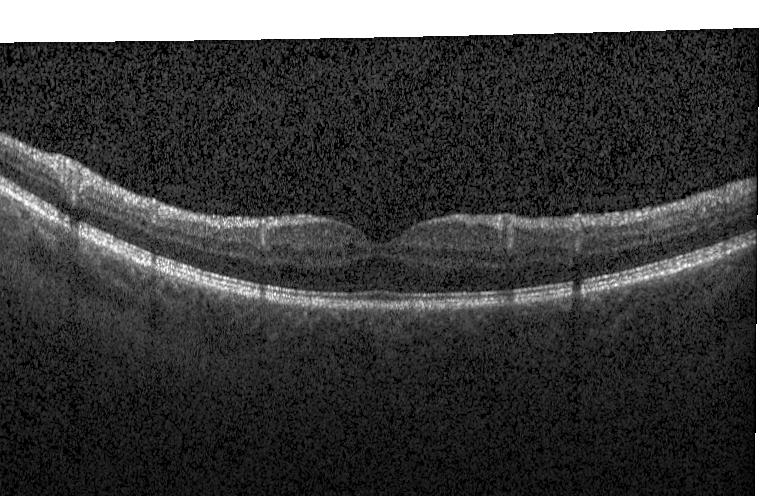

Diagnosis: no evidence of choroidal neovascularization, diabetic macular edema, or drusen.